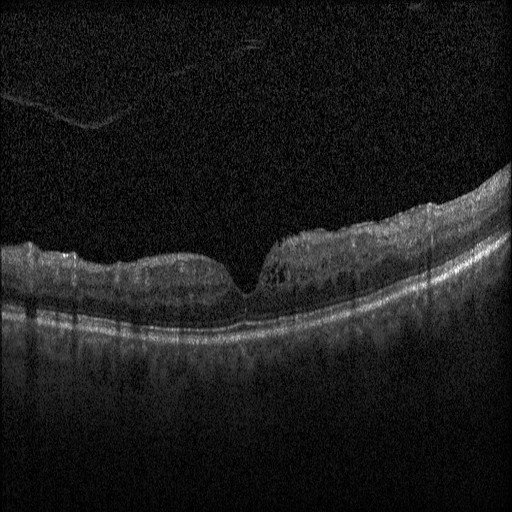
OCT B-scan.
Diabetic macular edema (DME).